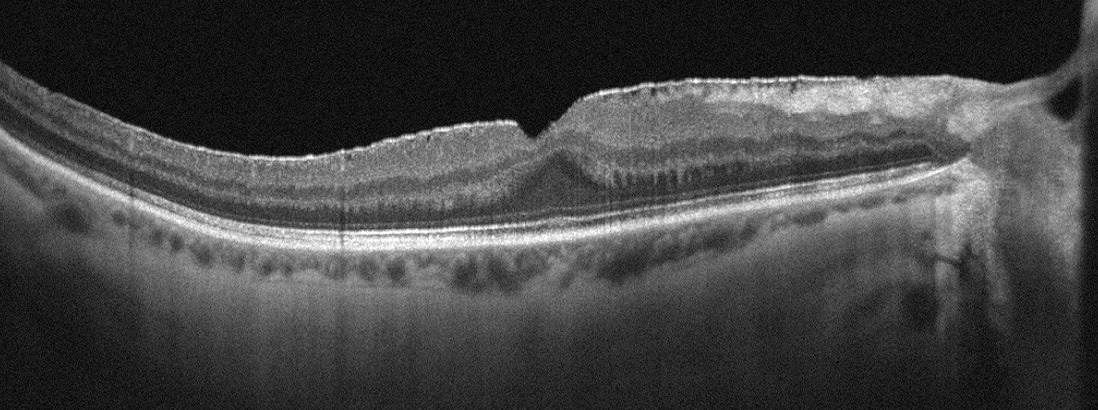

Optical coherence tomography scan
Epiretinal membrane (ERM).